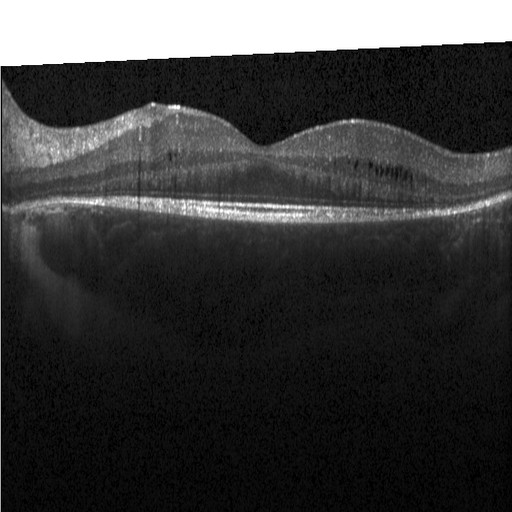 OCT line scan
Finding: DME.